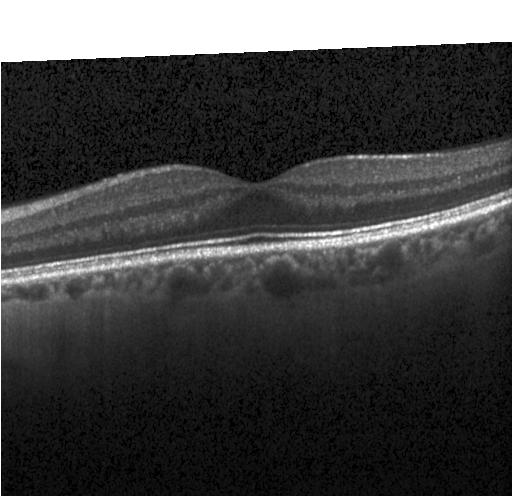
Instrument: Heidelberg Spectralis · optical coherence tomography B-scan · spectral-domain OCT.
Macular OCT: no evidence of choroidal neovascularization, diabetic macular edema, or drusen.